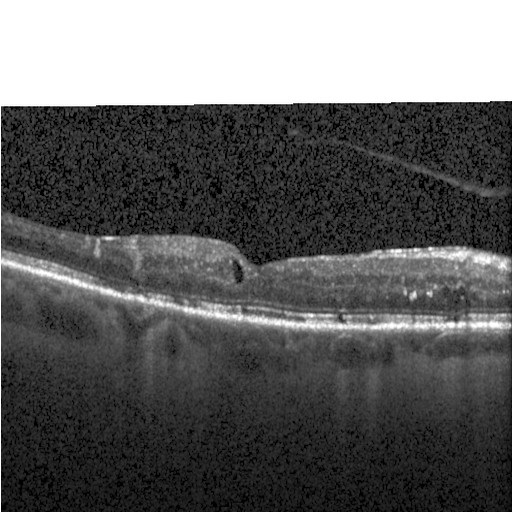 SD-OCT, retinal OCT B-scan, centered on the fovea — OCT finding: diabetic macular edema.